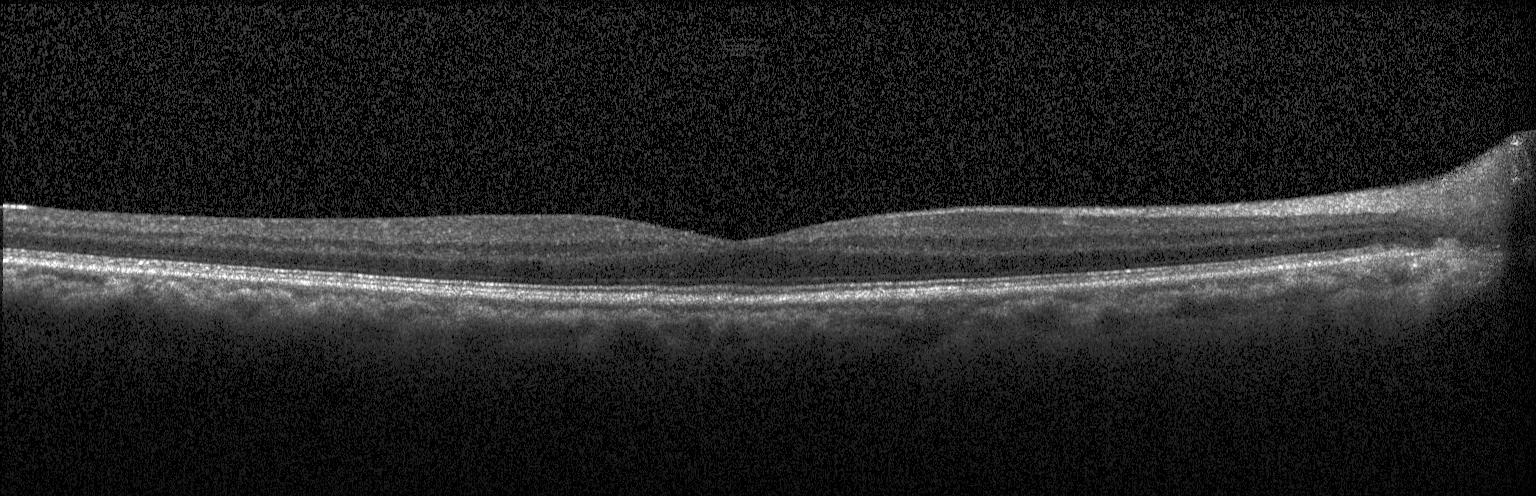 Horizontal scan through the fovea. Optical coherence tomography B-scan. Heidelberg Spectralis OCT system. OCT finding: neither choroidal neovascularization, diabetic macular edema, nor drusen.